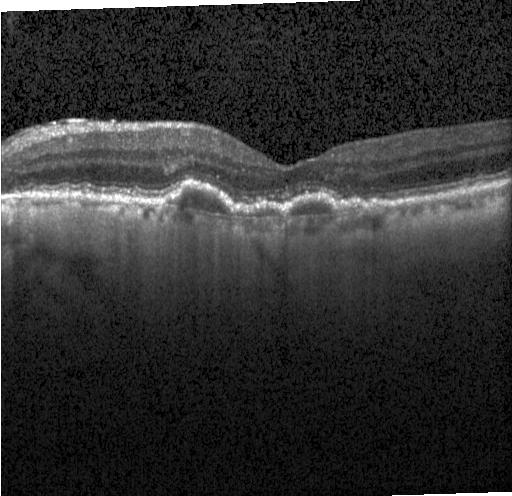 SD-OCT. Heidelberg Spectralis. Horizontal scan through the fovea. Retinal OCT cross-section. Finding: CNV.